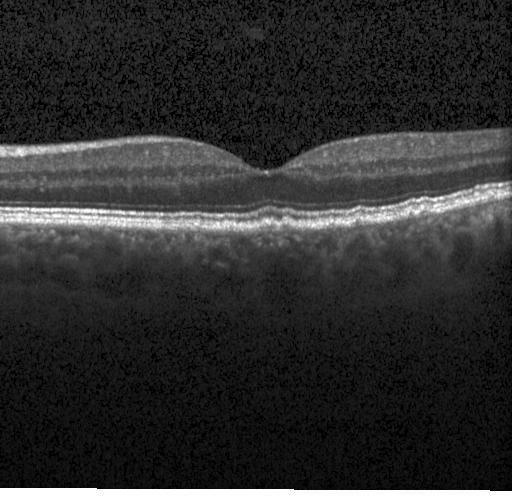 SD-OCT. OCT B-scan. Impression: drusen.